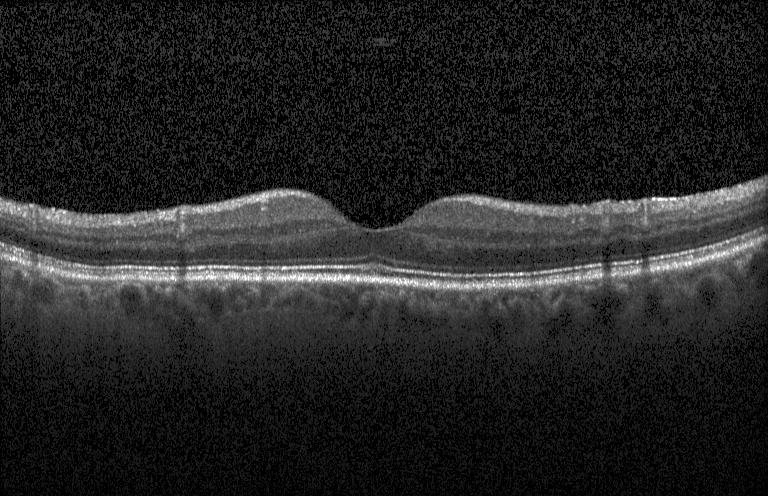
Macular OCT demonstrating no evidence of choroidal neovascularization, diabetic macular edema, or drusen.